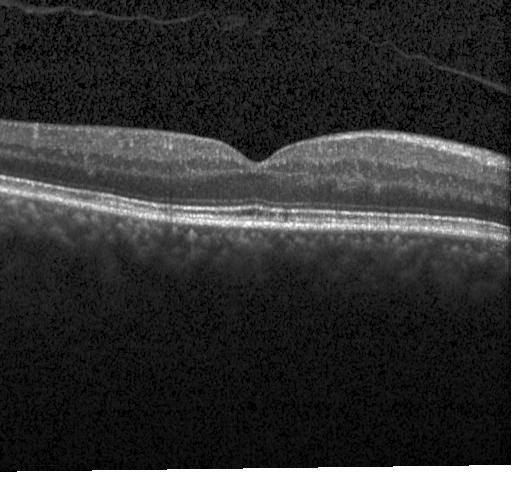 OCT B-scan
Finding: no evidence of CNV, DME, or drusen.